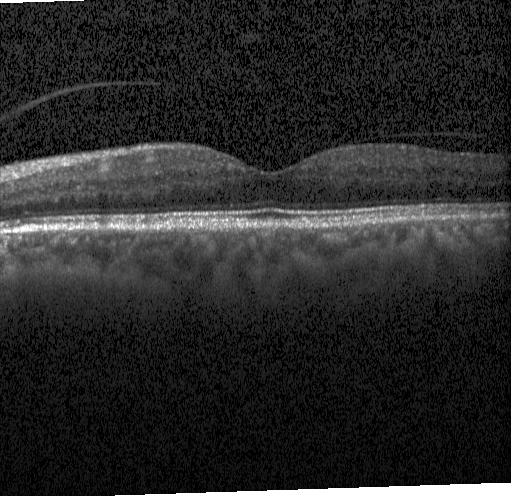

Spectral-domain optical coherence tomography. Macular scan. OCT B-scan. Diagnosis: no evidence of choroidal neovascularization, diabetic macular edema, or drusen.